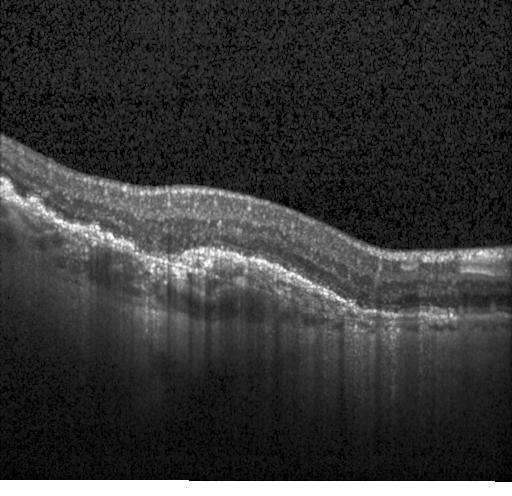

This B-scan demonstrates a choroidal neovascular membrane.